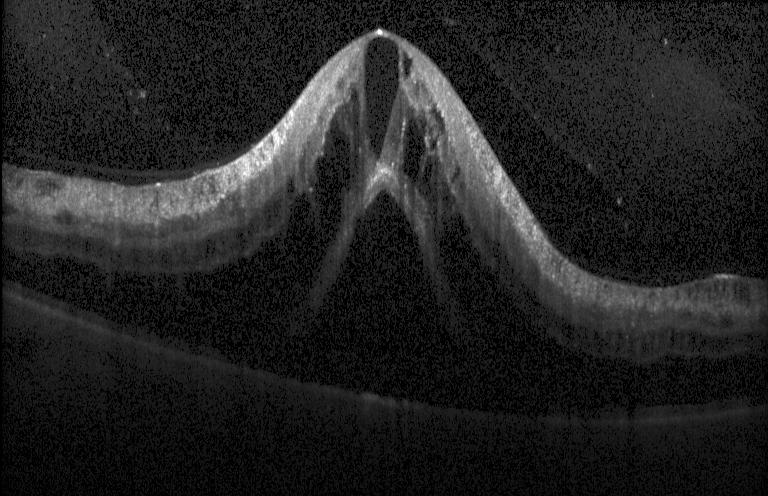

Macular scan, acquired on a Heidelberg Spectralis, retinal OCT cross-section, SD-OCT.
Dx: diabetic macular edema.